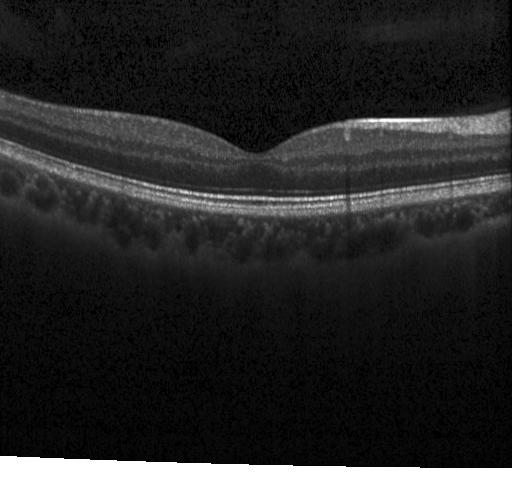
This B-scan demonstrates no evidence of CNV, DME, or drusen.